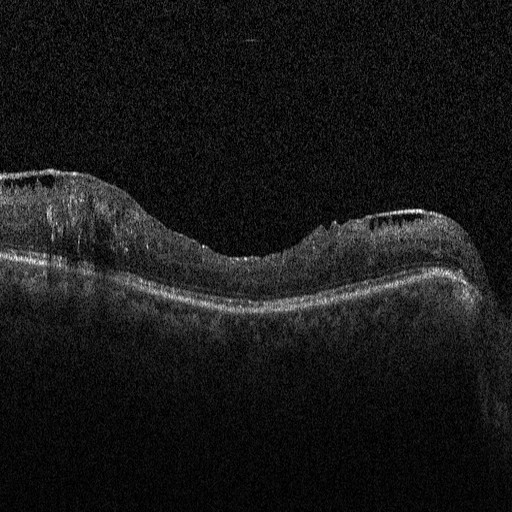 This B-scan demonstrates diabetic macular edema (DME).